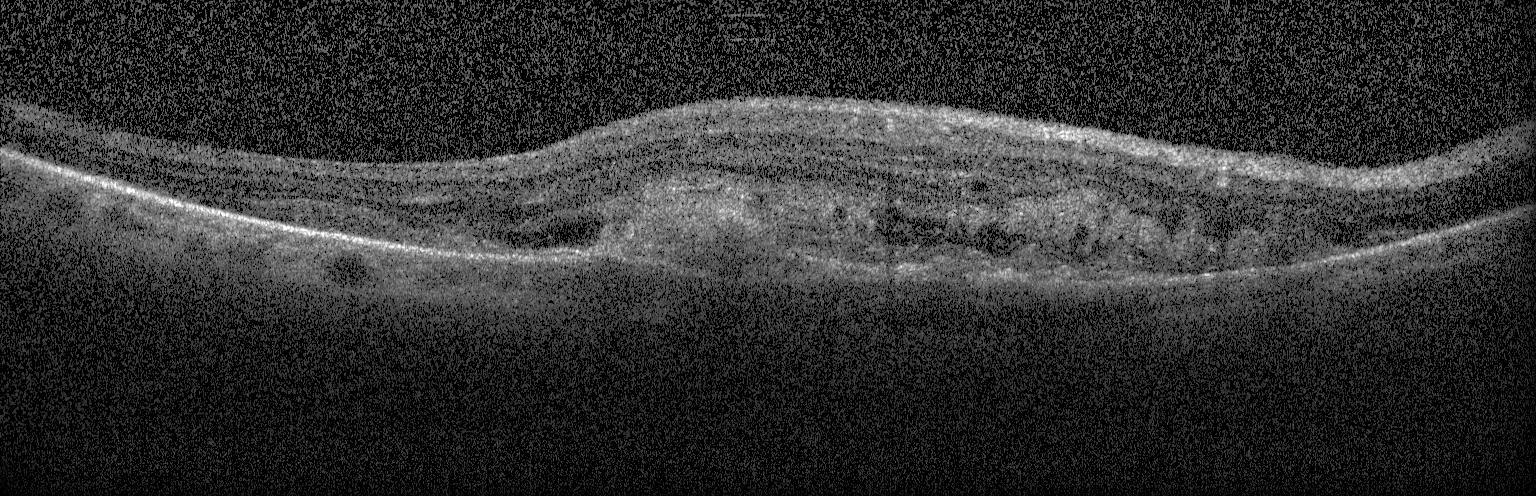 Heidelberg Spectralis OCT system. Spectral-domain OCT. Horizontal scan through the fovea. Optical coherence tomography B-scan. Macular OCT: CNV.